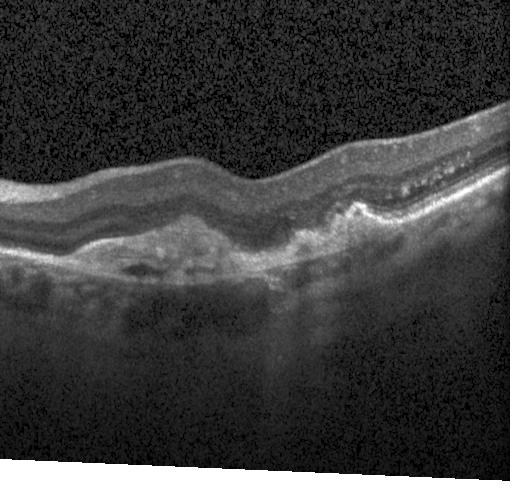
SD-OCT; retinal OCT B-scan
CNV.